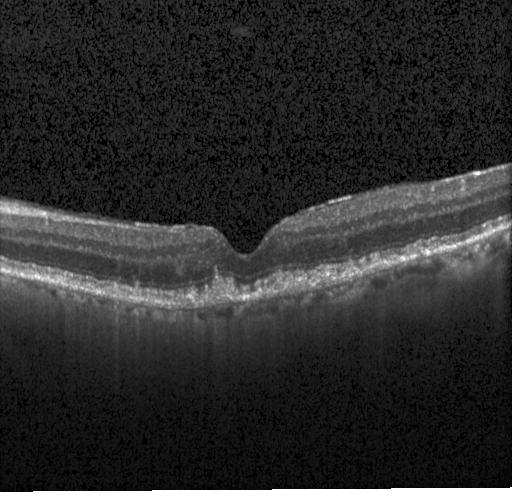 Optical coherence tomography scan. SD-OCT. Centered on the fovea.
Dx: multiple drusen.